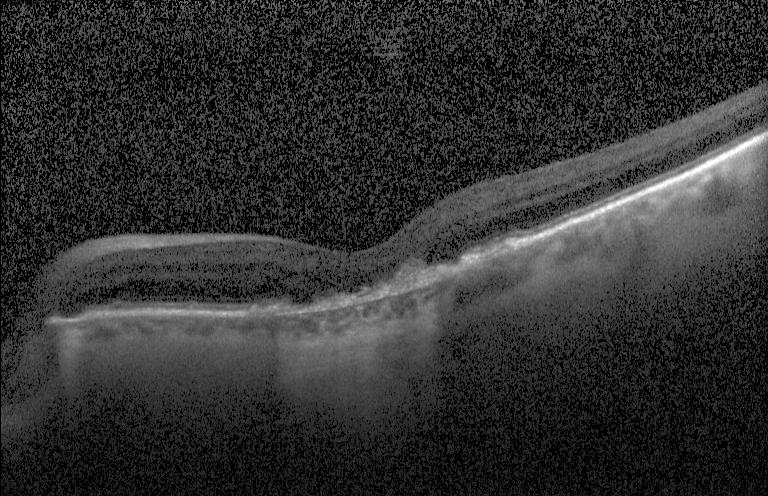 OCT scan showing a choroidal neovascular membrane.